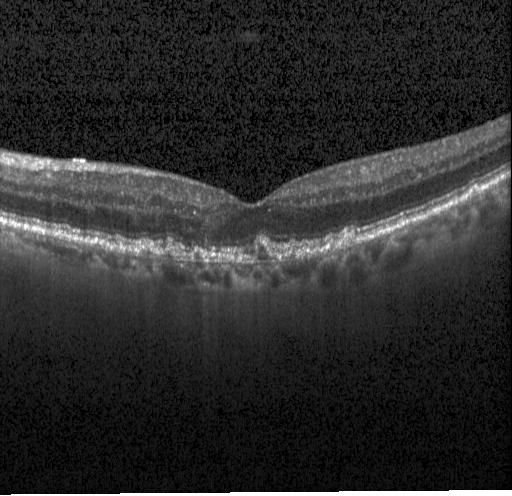
The scan shows choroidal neovascularization (CNV).